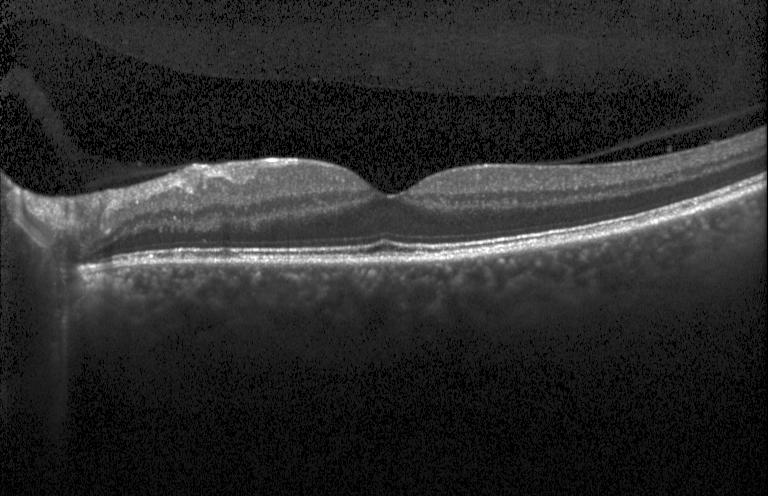
OCT line scan · Heidelberg Spectralis OCT system
No evidence of CNV, DME, or drusen.